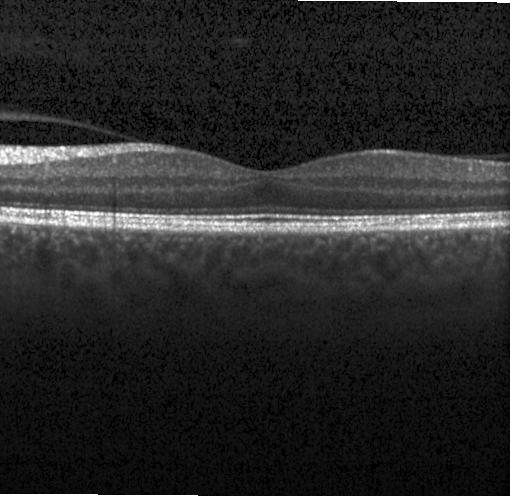

Spectral-domain optical coherence tomography, retinal OCT B-scan, horizontal scan through the fovea, instrument: Heidelberg Spectralis.
Diagnosis: no evidence of CNV, DME, or drusen.